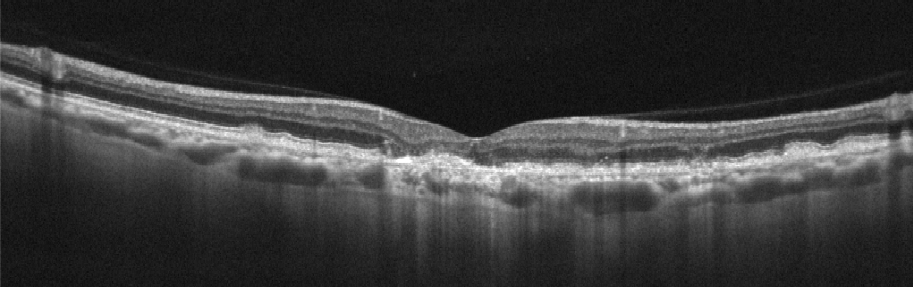
Optical coherence tomography B-scan.
Diagnosis: age-related macular degeneration (AMD).